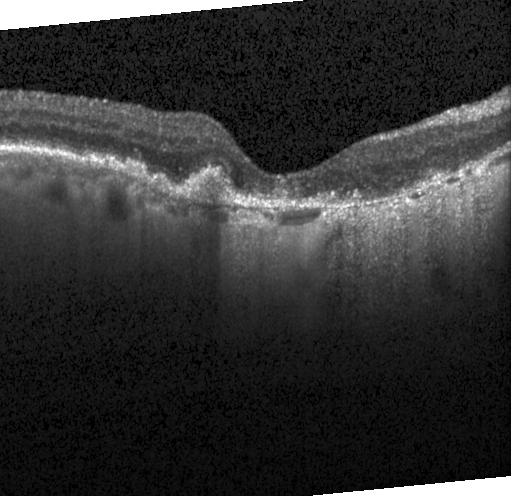 Macular OCT demonstrating a choroidal neovascular membrane.